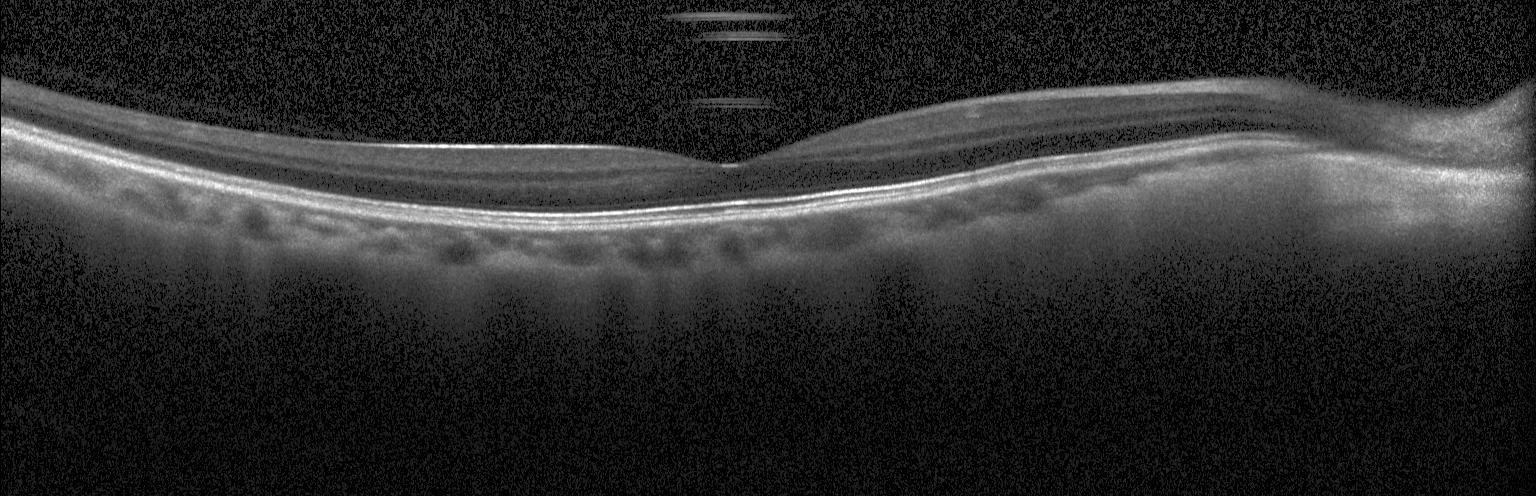
Retinal OCT cross-section.
Diagnosis: neither CNV, DME, nor drusen.